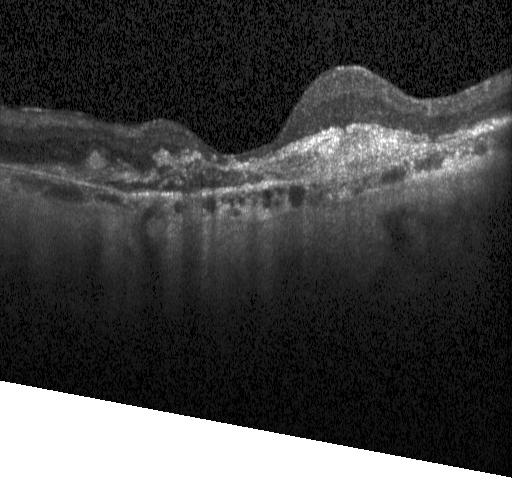
Spectral-domain OCT; OCT line scan — The scan shows a choroidal neovascular membrane.